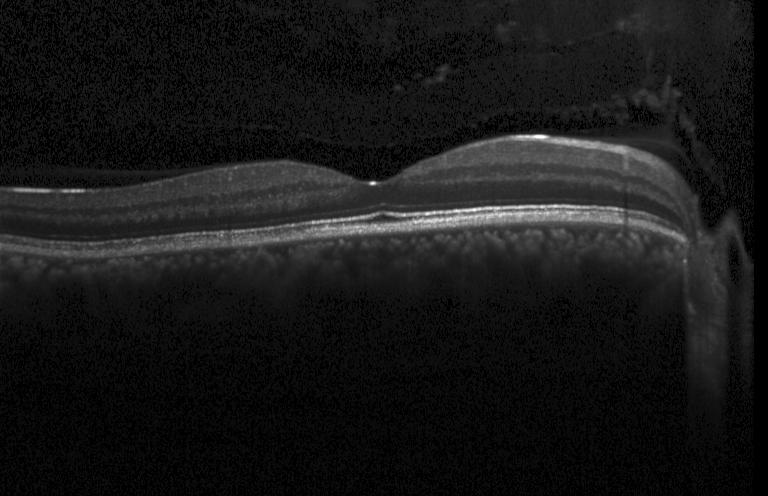
Finding: no choroidal neovascularization, no diabetic macular edema, and no drusen.